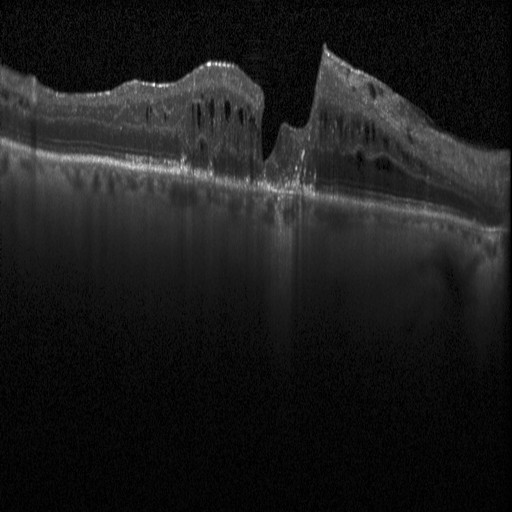 Retinal OCT B-scan. Impression: diabetic macular edema (DME).